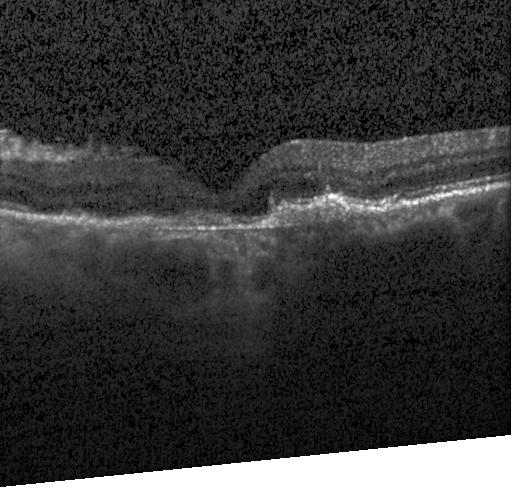

Assessment: choroidal neovascularization.